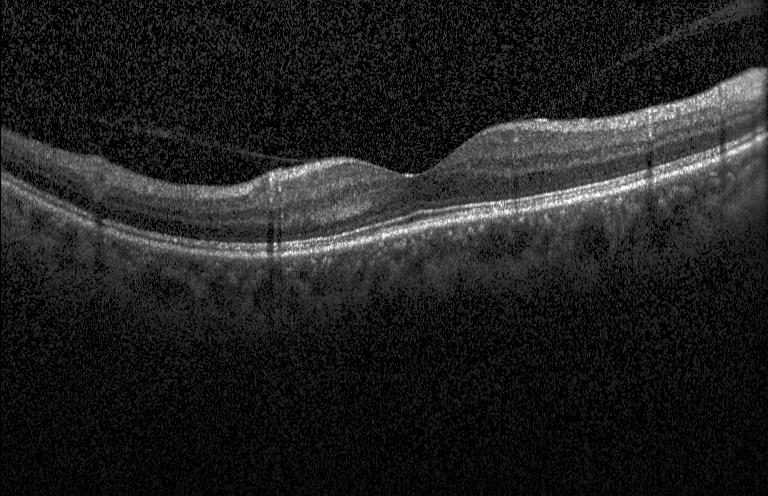
Retinal OCT cross-section showing neither choroidal neovascularization, diabetic macular edema, nor drusen.